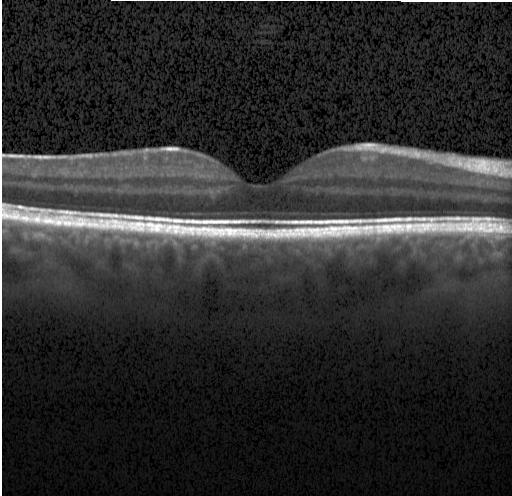 OCT B-scan. SD-OCT. Through the macula — The scan shows neither choroidal neovascularization, diabetic macular edema, nor drusen.